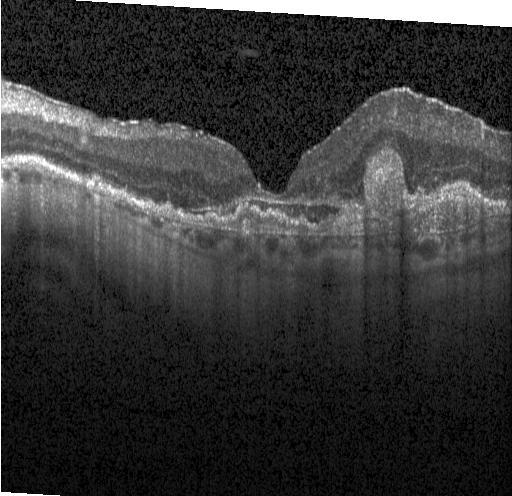

Retinal OCT cross-section. The scan shows CNV.